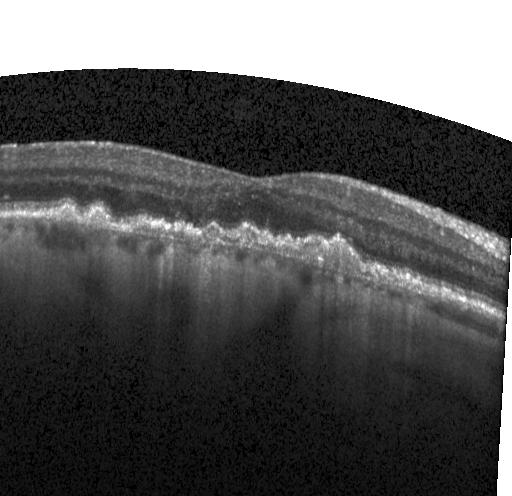

Retinal OCT B-scan. Dx: CNV.